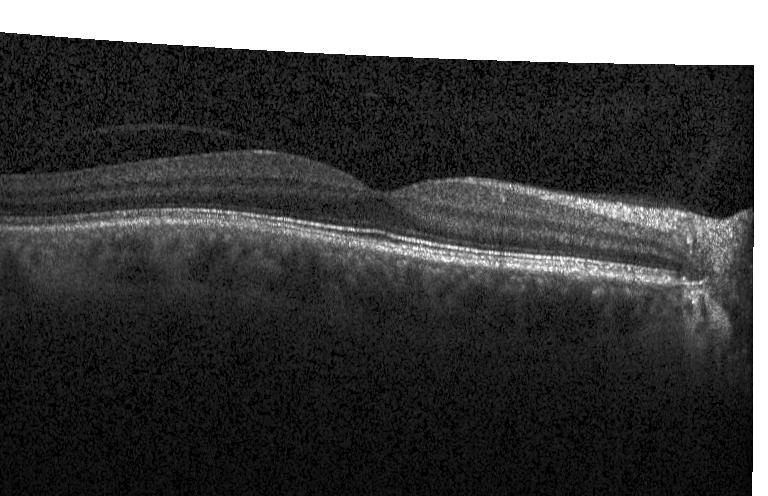

Spectral-domain OCT B-scan: neither choroidal neovascularization, diabetic macular edema, nor drusen.